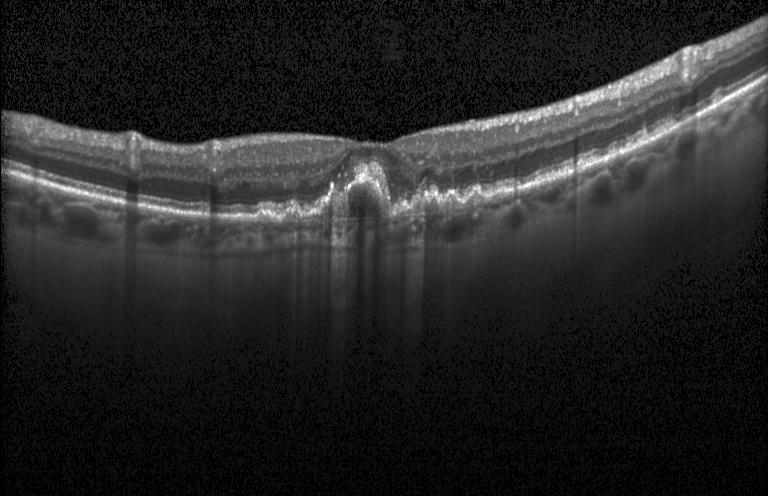
Spectral-domain OCT, Heidelberg Spectralis OCT system, through the macula, OCT line scan
Diagnosis: choroidal neovascularization.